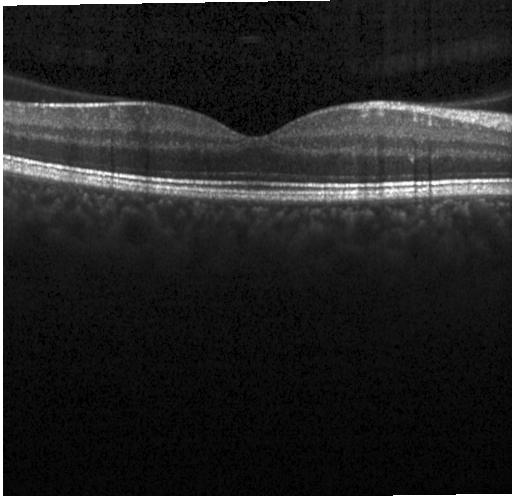

Optical coherence tomography scan. No evidence of choroidal neovascularization, diabetic macular edema, or drusen.